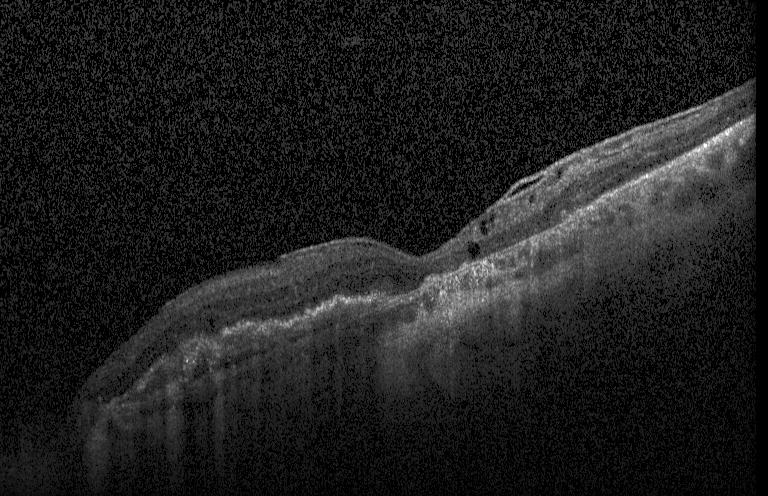
The scan shows choroidal neovascularization.